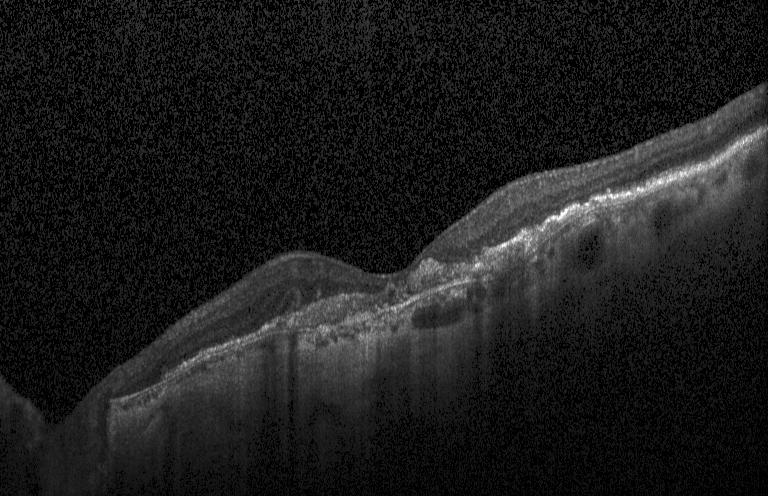

Heidelberg Spectralis, horizontal scan through the fovea, optical coherence tomography scan, spectral-domain OCT.
Assessment: choroidal neovascularization.